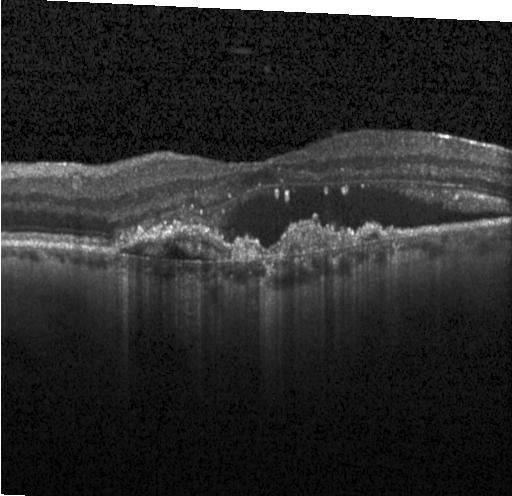

Optical coherence tomography scan, spectral-domain optical coherence tomography, Heidelberg Spectralis OCT system, through the macula — Diagnosis: choroidal neovascularization (CNV).